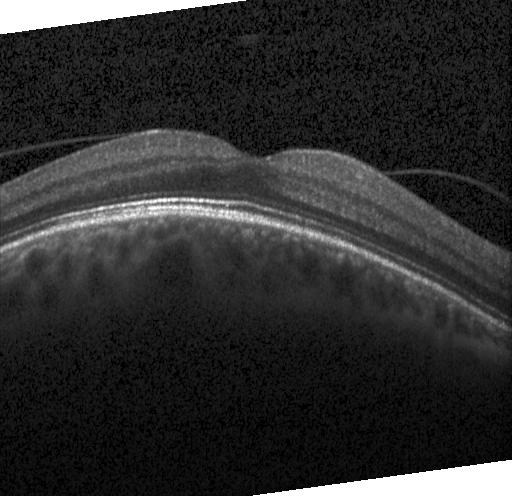
OCT B-scan showing no CNV, no DME, and no drusen.